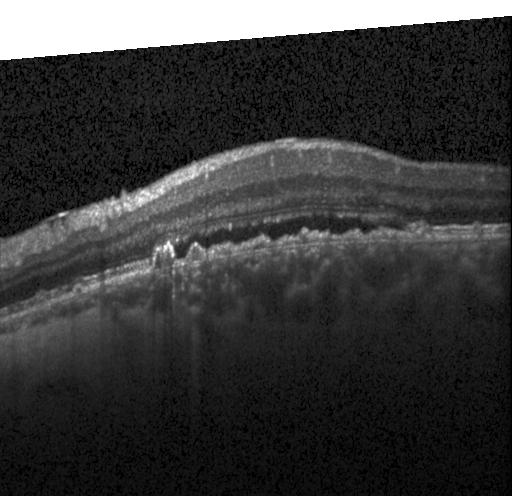

Impression: CNV.